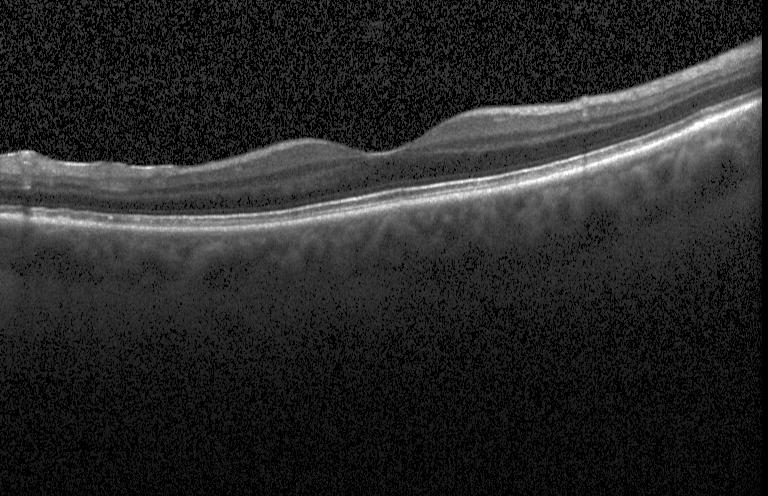

Macular OCT demonstrating no evidence of CNV, DME, or drusen.